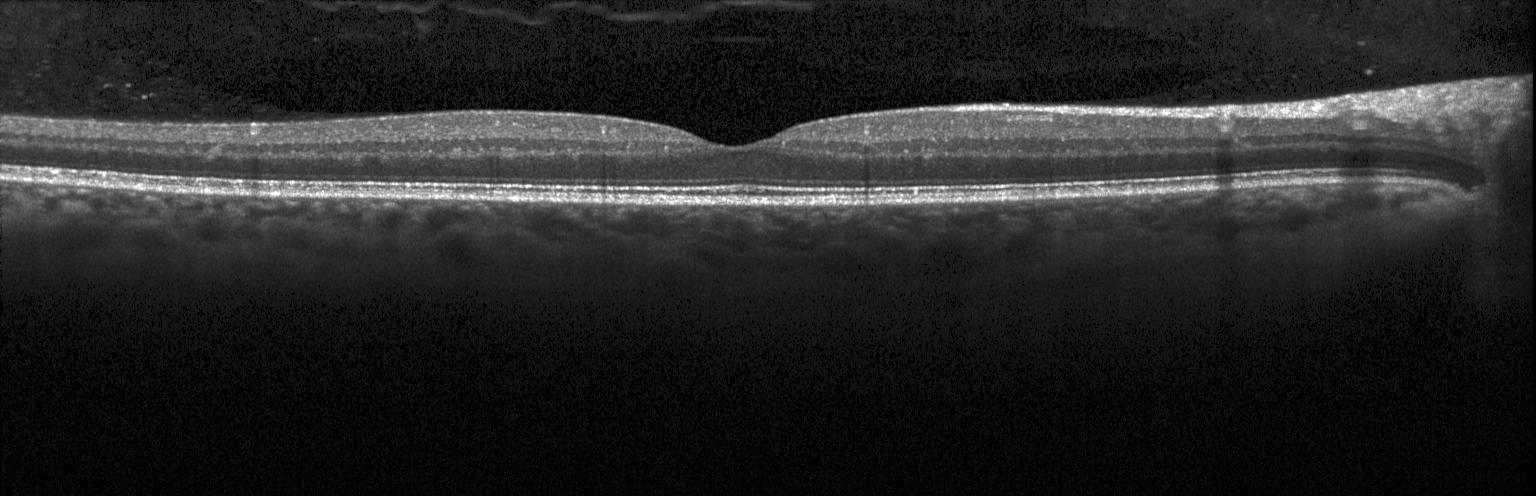 OCT B-scan. Impression: no choroidal neovascularization, no diabetic macular edema, and no drusen.